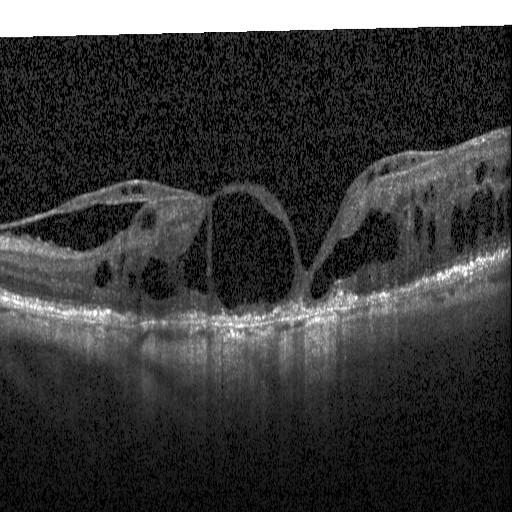

This B-scan demonstrates diabetic macular edema (DME).